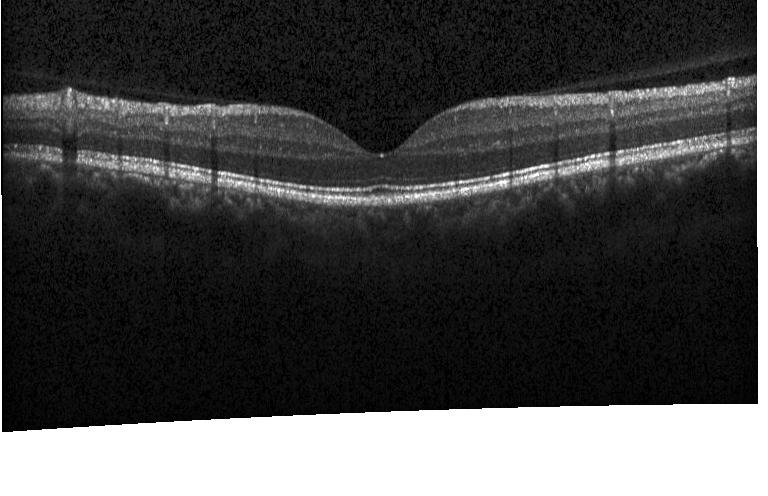
Impression: no choroidal neovascularization, diabetic macular edema, or drusen.